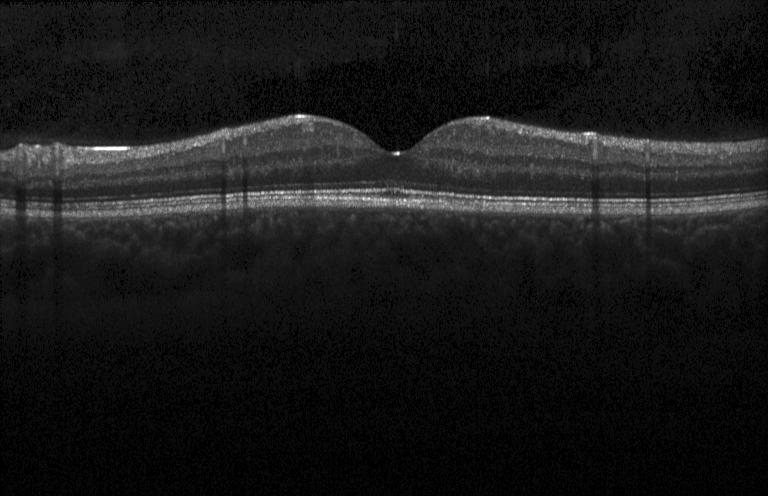
OCT line scan. Centered on the fovea. This B-scan demonstrates neither choroidal neovascularization, diabetic macular edema, nor drusen.